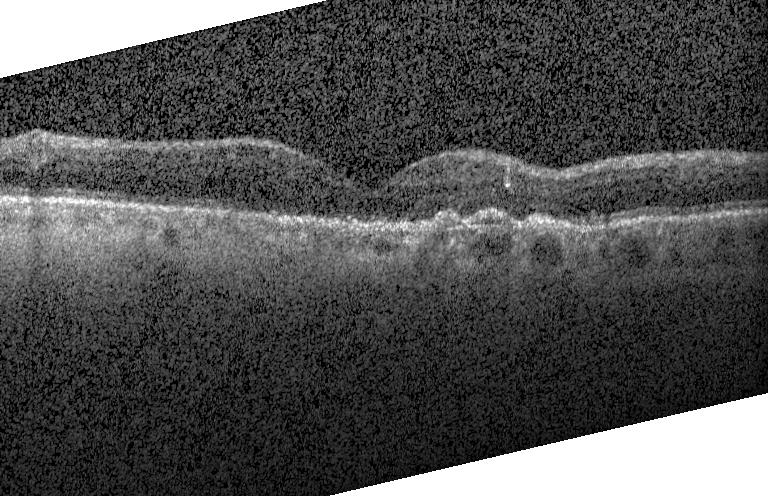

Finding: a choroidal neovascular membrane.